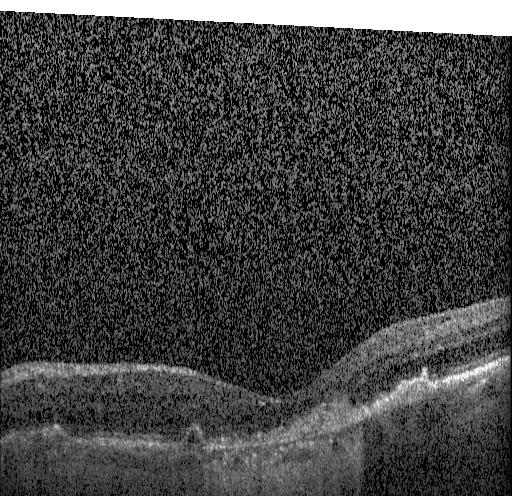

Retinal OCT B-scan · spectral-domain optical coherence tomography · centered on the fovea
Impression: a choroidal neovascular membrane.